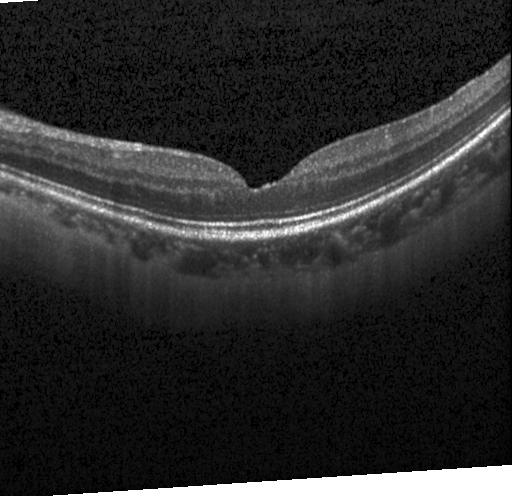 Impression: no evidence of choroidal neovascularization, diabetic macular edema, or drusen.